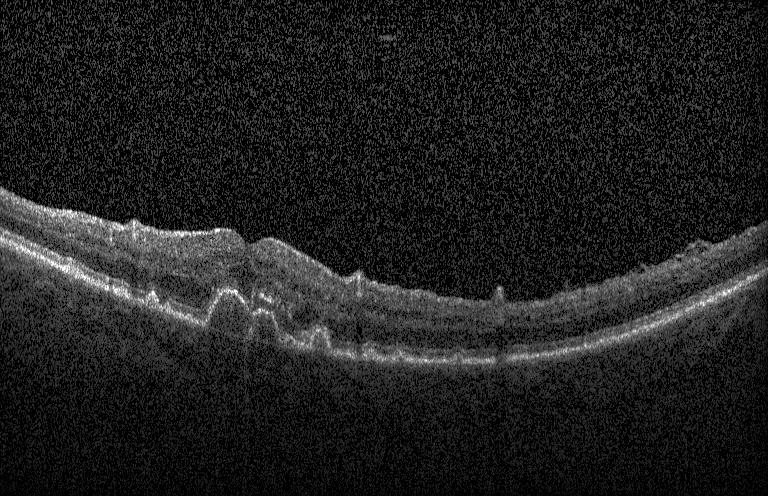
Macular scan. Heidelberg Spectralis OCT system. SD-OCT. Optical coherence tomography B-scan — Finding: drusen.